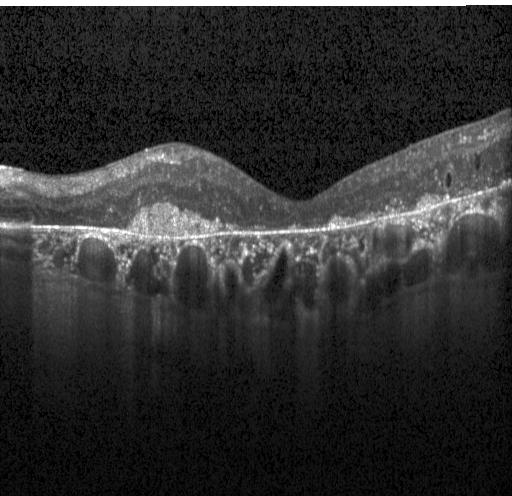

SD-OCT; instrument: Heidelberg Spectralis; horizontal scan through the fovea; OCT B-scan. Finding: choroidal neovascularization.